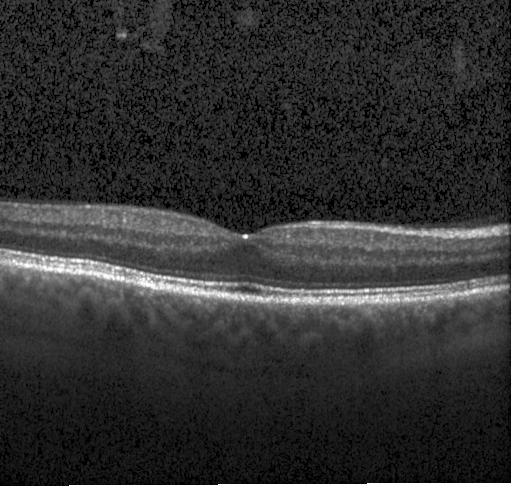 Optical coherence tomography scan — This B-scan demonstrates neither choroidal neovascularization, diabetic macular edema, nor drusen.